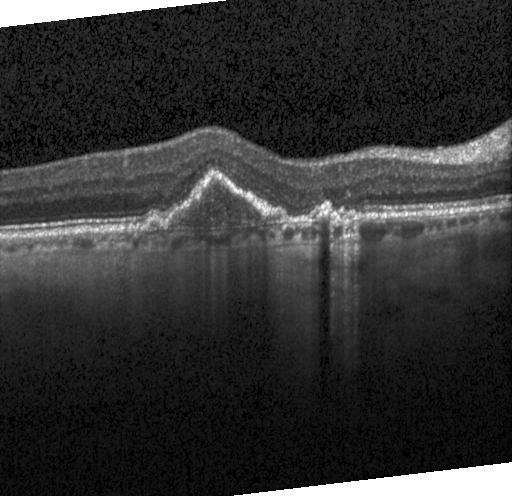
Macular OCT demonstrating a choroidal neovascular membrane.